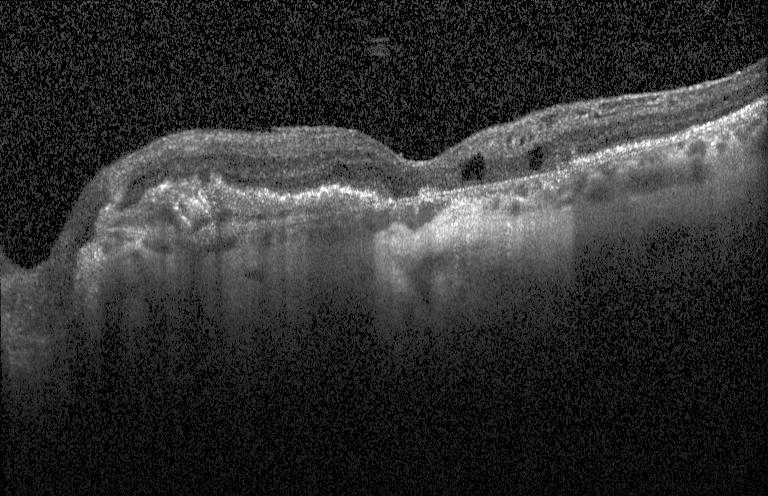 Retinal OCT B-scan. Instrument: Heidelberg Spectralis. Dx: choroidal neovascularization.